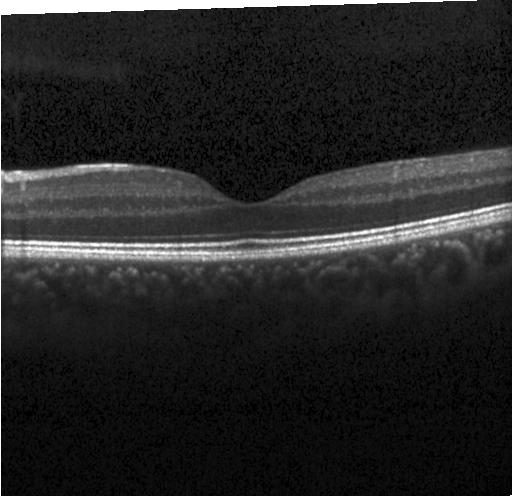
Through the macula, OCT line scan. Assessment: no choroidal neovascularization, diabetic macular edema, or drusen.